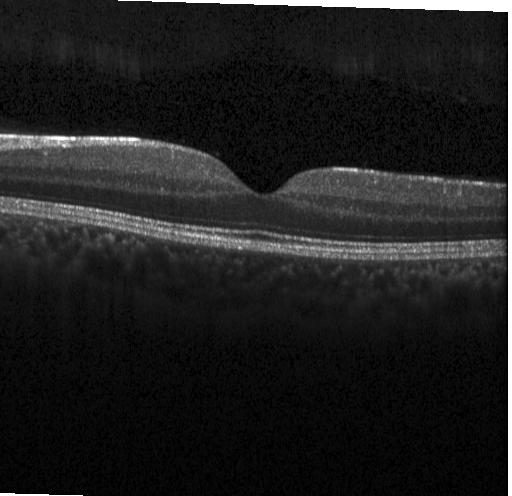

Diagnosis: no CNV, no DME, and no drusen.